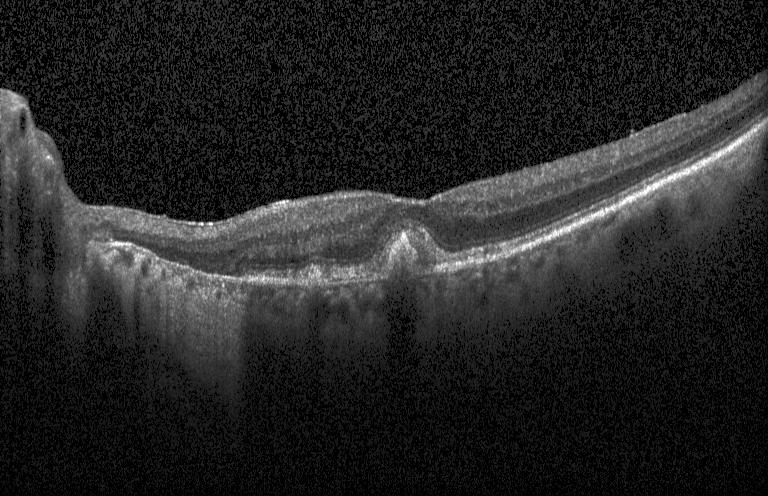

Heidelberg Spectralis OCT system; optical coherence tomography B-scan; SD-OCT; through the macula. The scan shows CNV.